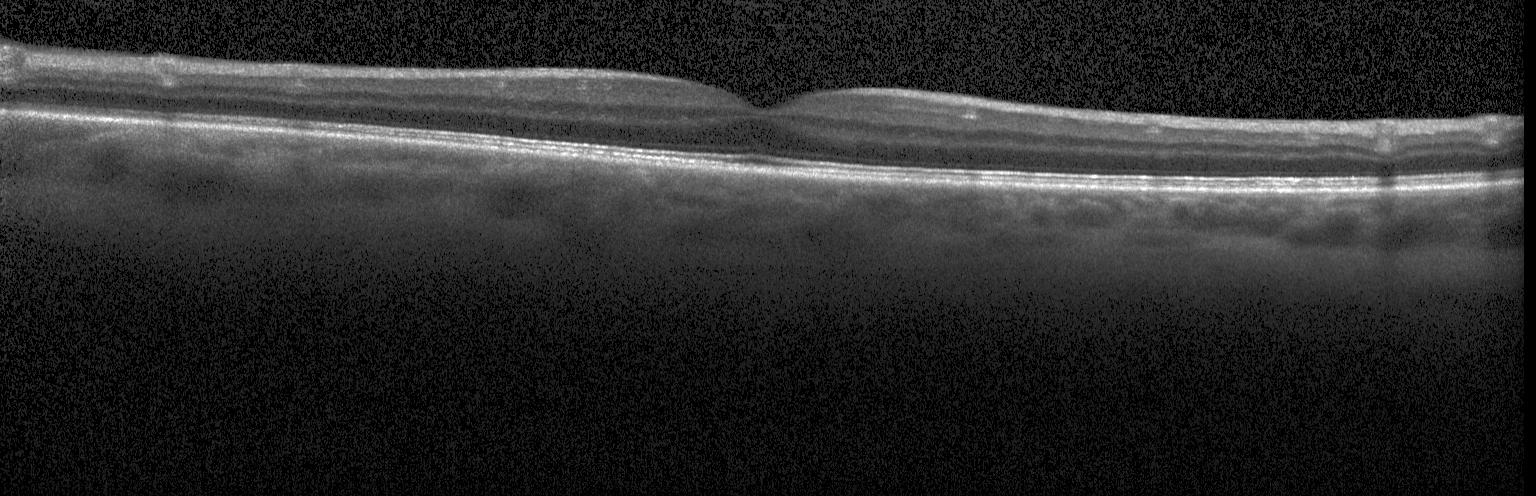 Acquired on a Heidelberg Spectralis; spectral-domain optical coherence tomography; retinal OCT cross-section — Macular OCT: neither CNV, DME, nor drusen.